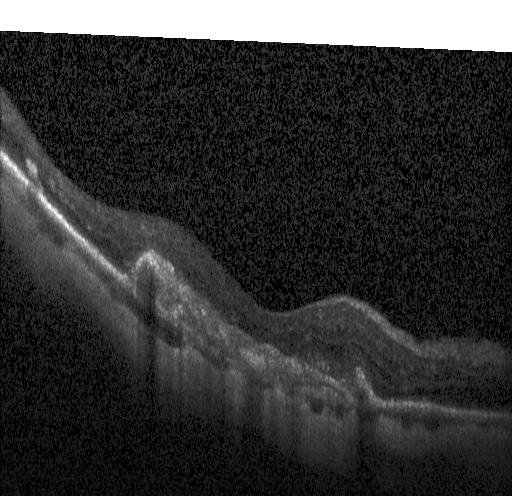 Assessment: choroidal neovascularization (CNV).